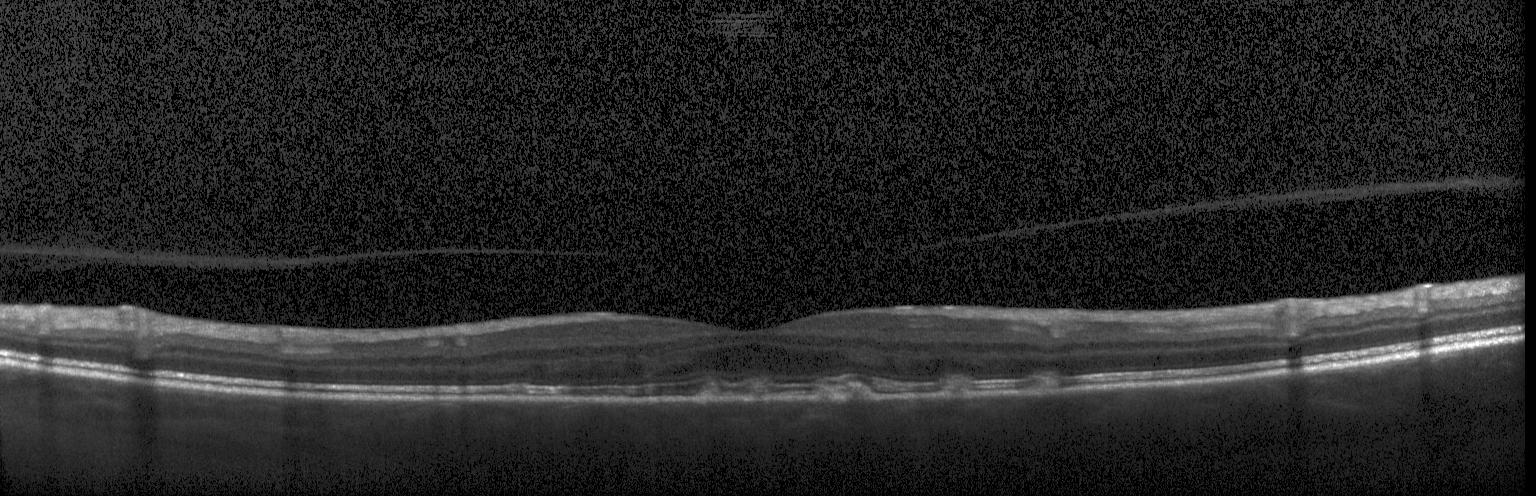

SD-OCT, fovea-centered, optical coherence tomography B-scan, Heidelberg Spectralis. Impression: drusen.